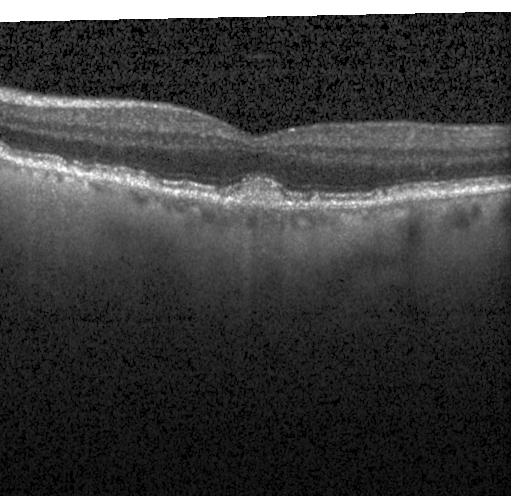
Spectral-domain optical coherence tomography. Instrument: Heidelberg Spectralis. OCT line scan — Impression: drusen.